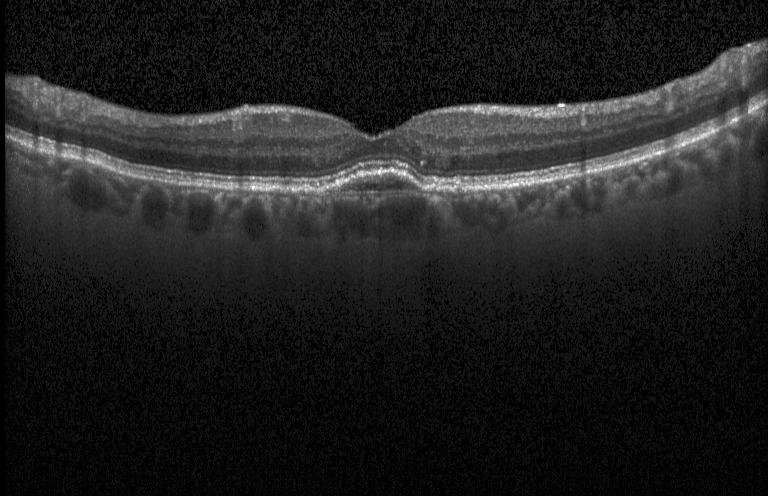
Spectral-domain OCT B-scan: choroidal neovascularization.